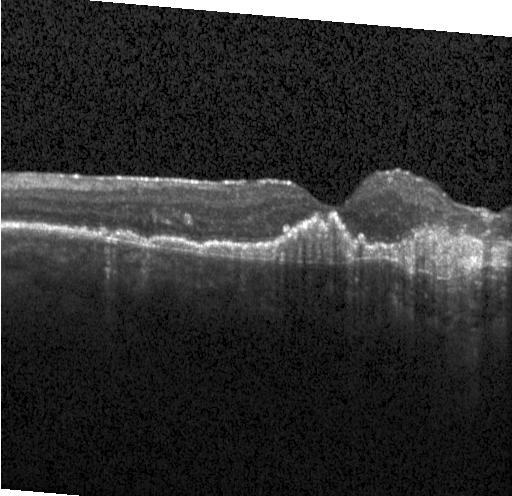

OCT B-scan showing CNV.